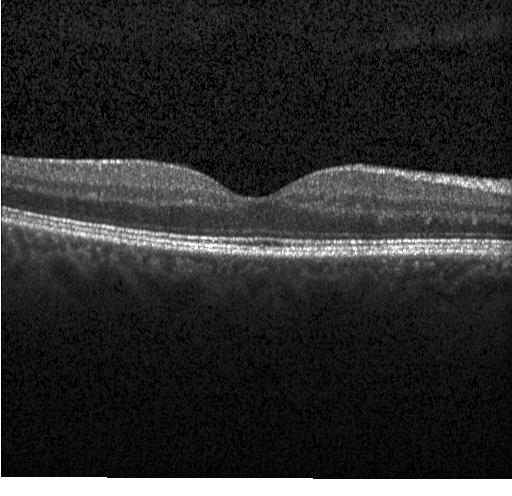

Instrument: Heidelberg Spectralis, retinal OCT cross-section, fovea-centered — The scan shows neither choroidal neovascularization, diabetic macular edema, nor drusen.